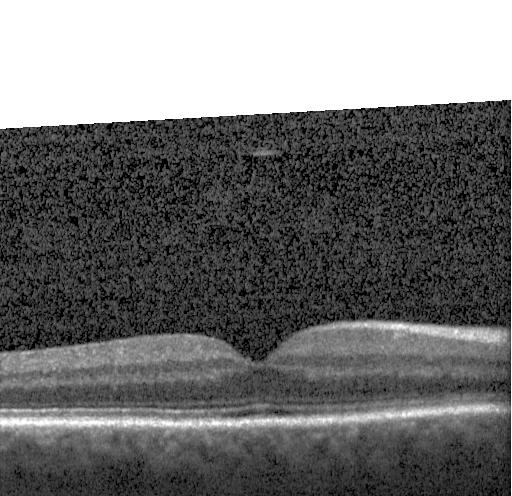

Macular OCT demonstrating no CNV, no DME, and no drusen.